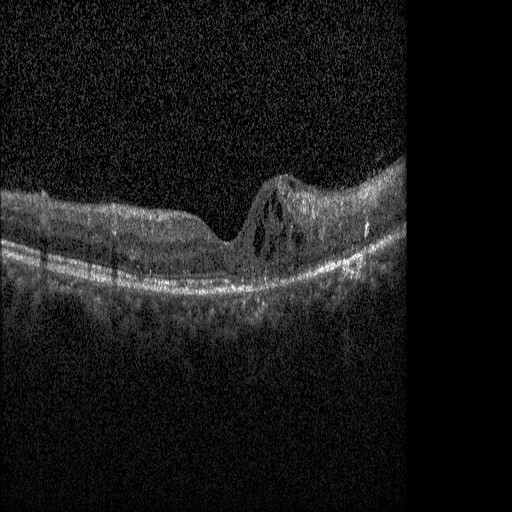
Spectral-domain optical coherence tomography; centered on the fovea; instrument: Heidelberg Spectralis; retinal OCT cross-section
Diabetic macular edema (DME).